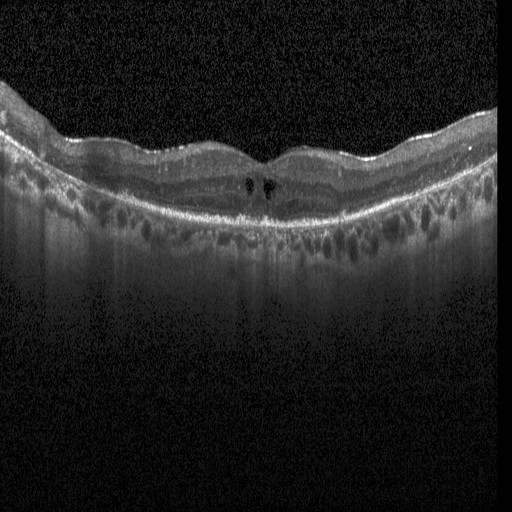 Spectral-domain OCT. Retinal OCT B-scan. Centered on the fovea.
Finding: diabetic macular edema.